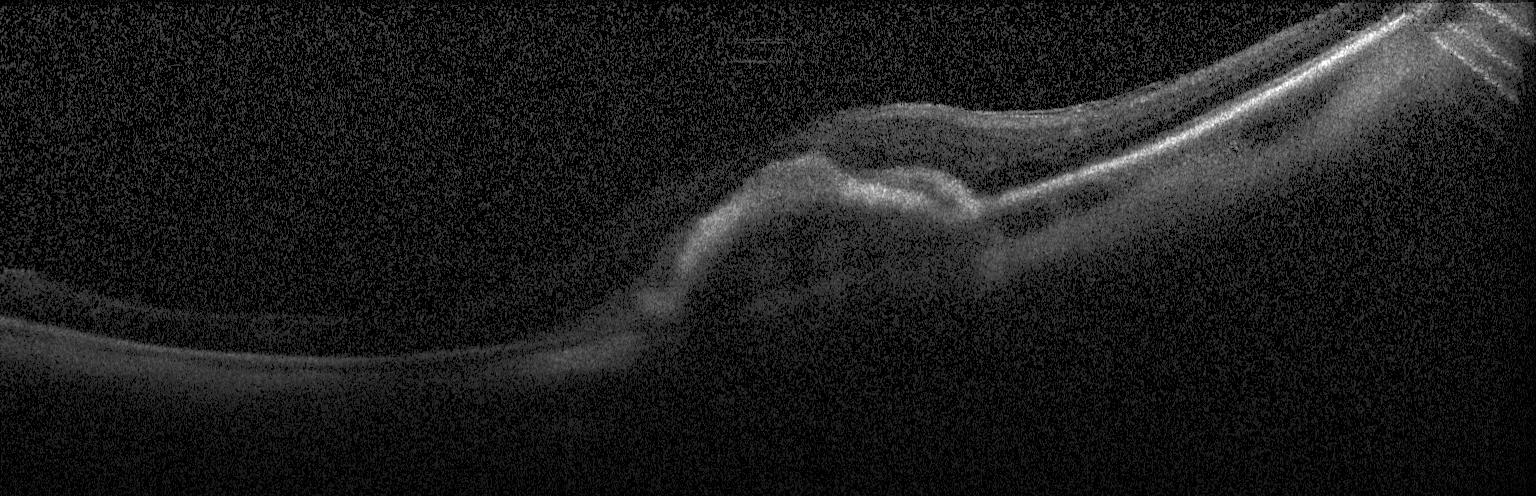 SD-OCT; OCT line scan — The scan shows a choroidal neovascular membrane.